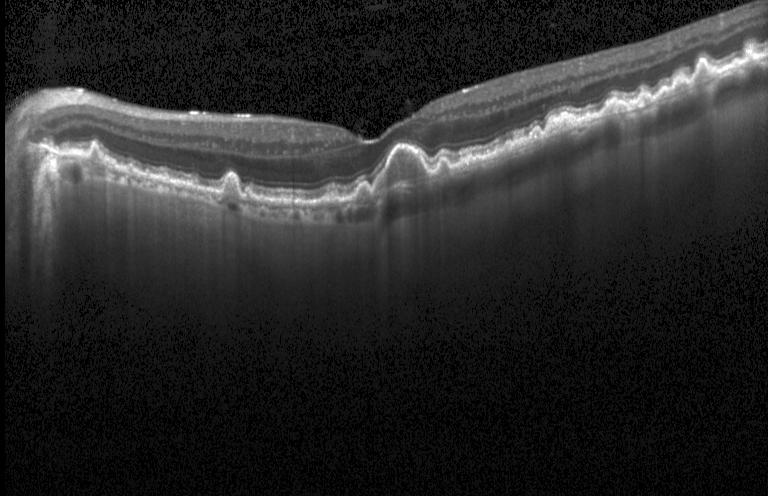

Optical coherence tomography scan. Heidelberg Spectralis OCT system. Fovea-centered. Spectral-domain OCT.
Diagnosis: drusen.